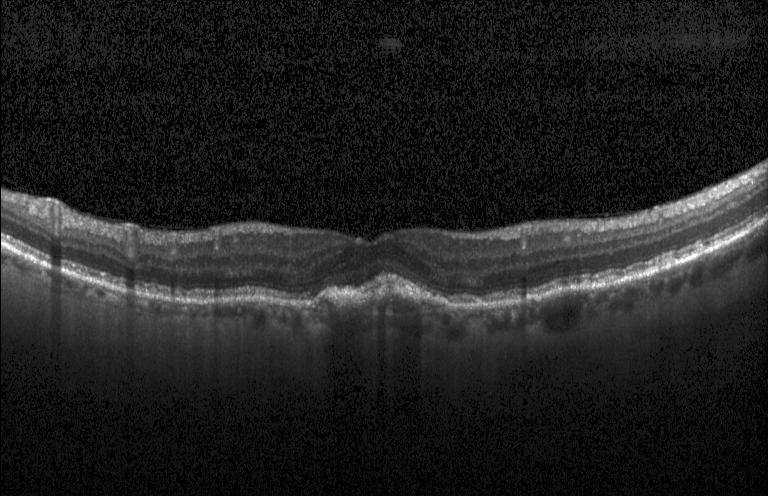
Retinal OCT cross-section.
The scan shows choroidal neovascularization.